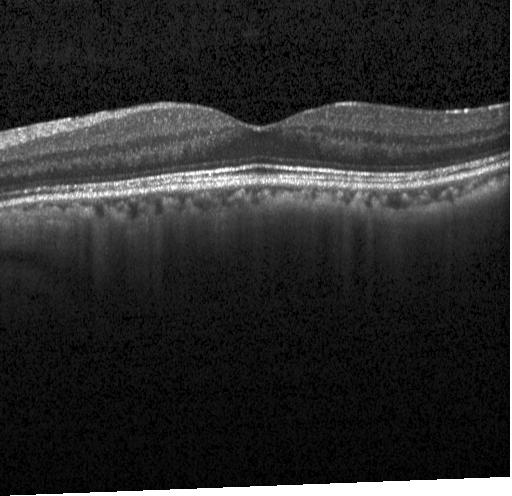 Heidelberg Spectralis OCT system · spectral-domain optical coherence tomography · horizontal scan through the fovea · OCT B-scan.
Impression: no choroidal neovascularization, no diabetic macular edema, and no drusen.